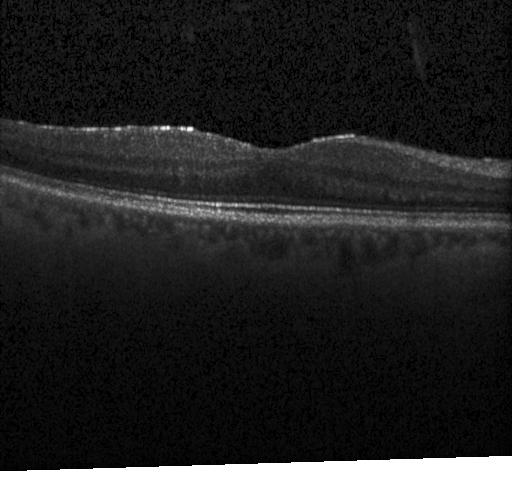

Optical coherence tomography B-scan.
No choroidal neovascularization, no diabetic macular edema, and no drusen.